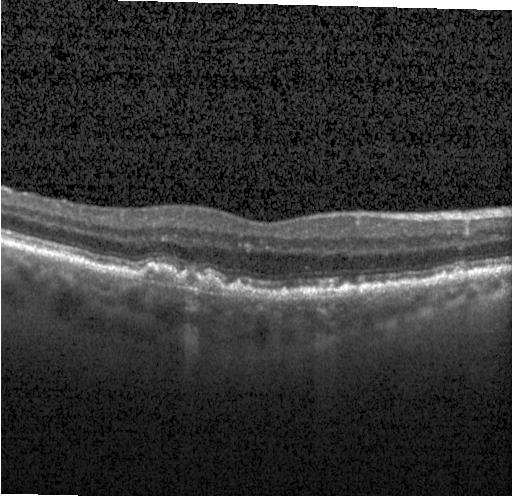
OCT B-scan — Diagnosis: drusen.